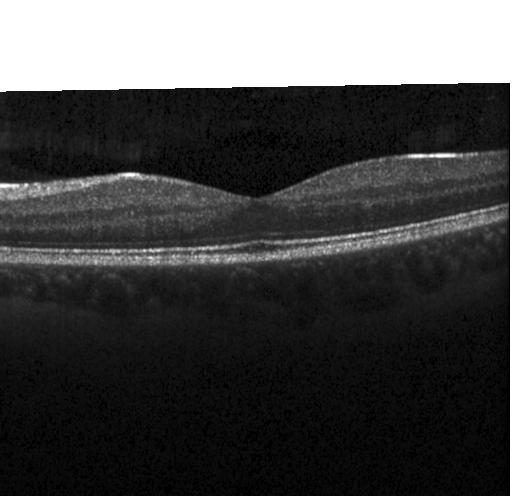

Retinal OCT B-scan; Heidelberg Spectralis; SD-OCT — Diagnosis: no CNV, no DME, and no drusen.